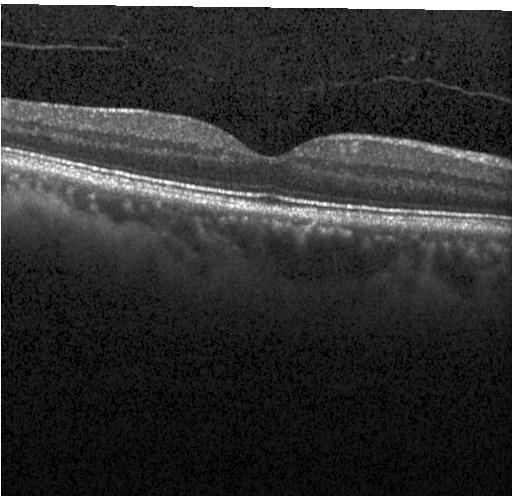 Through the macula. Retinal OCT B-scan. Instrument: Heidelberg Spectralis — Assessment: no evidence of choroidal neovascularization, diabetic macular edema, or drusen.